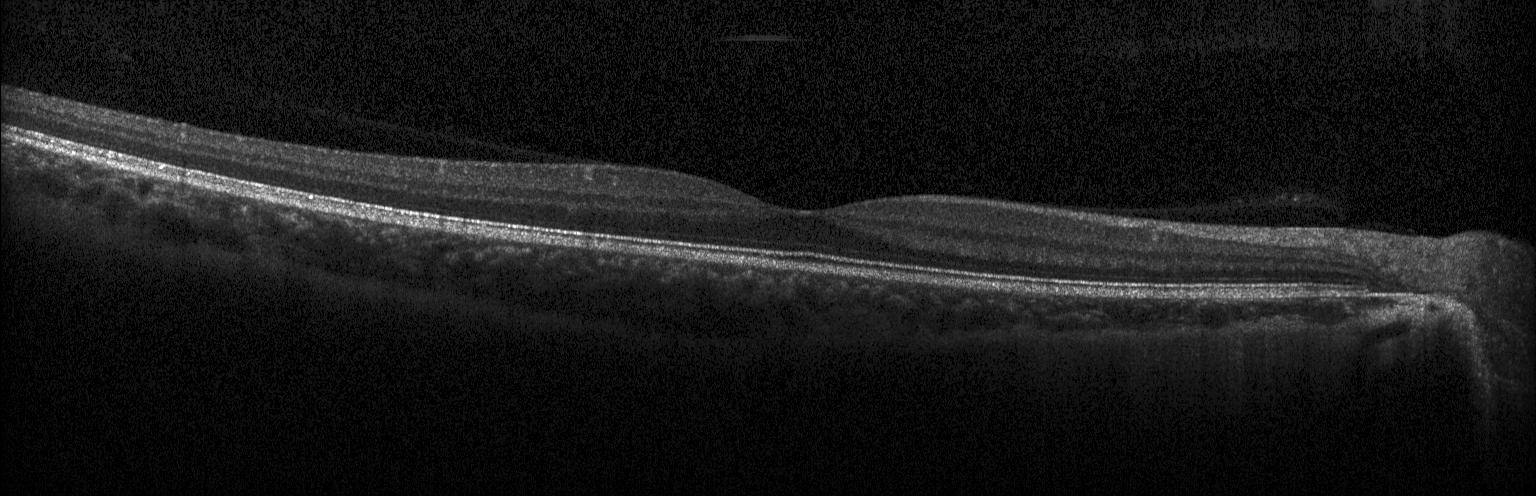

Horizontal scan through the fovea; optical coherence tomography B-scan
OCT finding: no evidence of choroidal neovascularization, diabetic macular edema, or drusen.